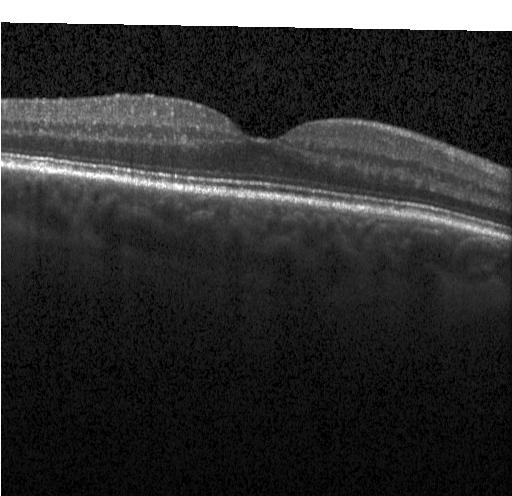 OCT line scan, spectral-domain optical coherence tomography. This B-scan demonstrates no choroidal neovascularization, diabetic macular edema, or drusen.